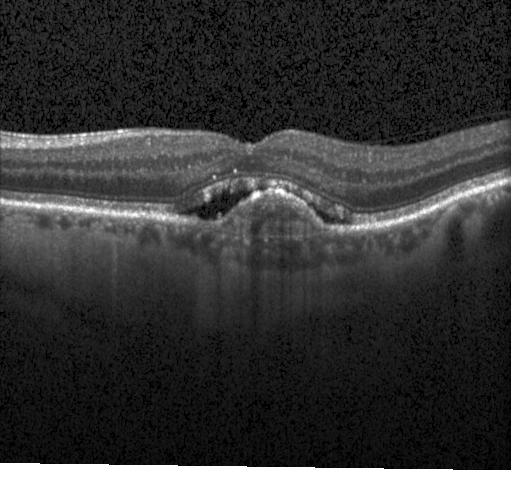 Acquired on a Heidelberg Spectralis · OCT line scan · spectral-domain optical coherence tomography.
Assessment: choroidal neovascularization.